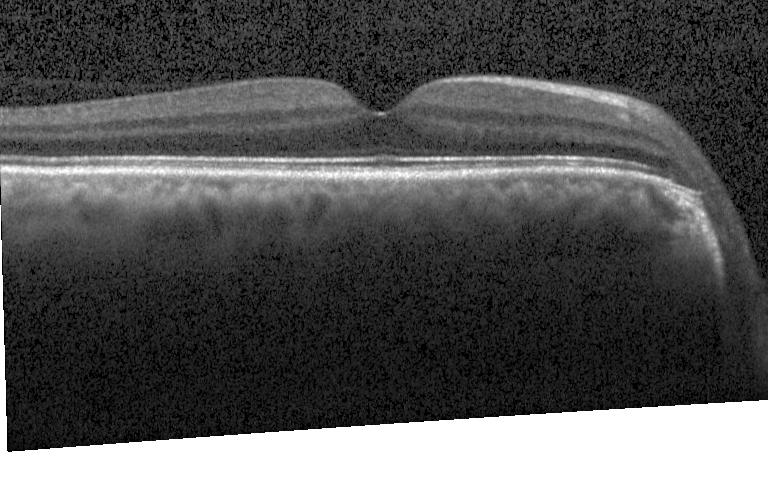 Assessment: no choroidal neovascularization, no diabetic macular edema, and no drusen.